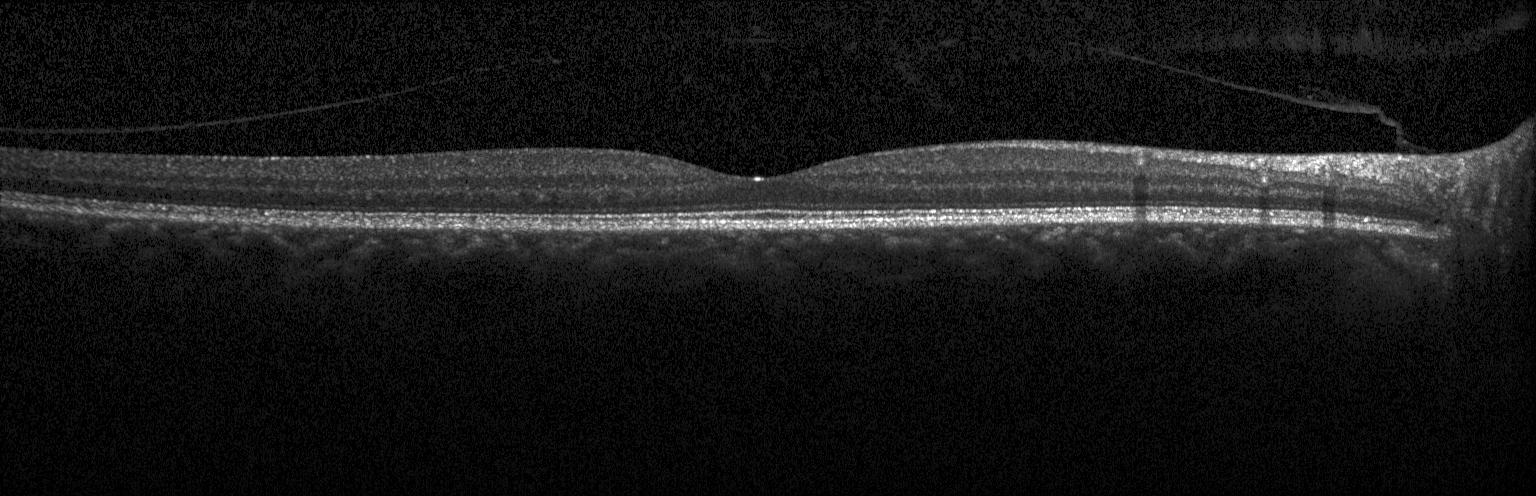
OCT B-scan, Heidelberg Spectralis, spectral-domain OCT — Impression: no choroidal neovascularization, diabetic macular edema, or drusen.